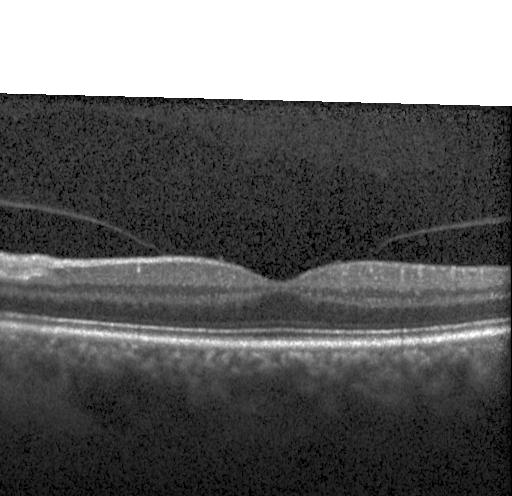

Retinal OCT B-scan, Heidelberg Spectralis OCT system — Impression: no choroidal neovascularization, diabetic macular edema, or drusen.